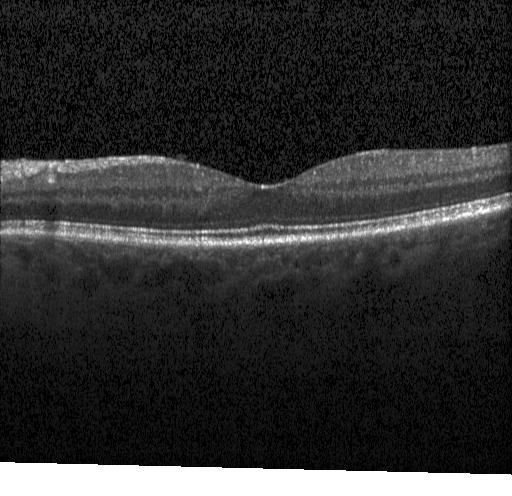 Dx: no choroidal neovascularization, diabetic macular edema, or drusen.